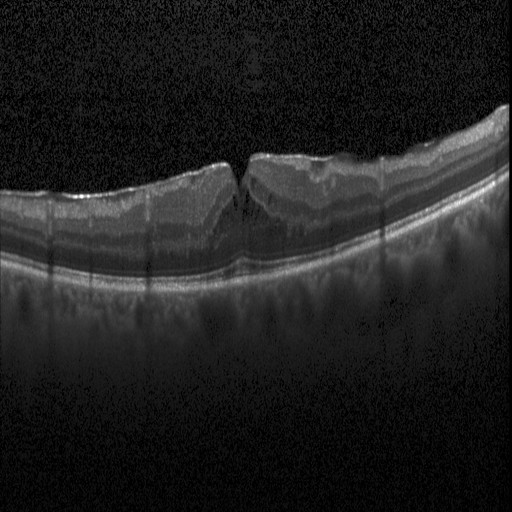

Retinal OCT cross-section — This B-scan demonstrates diabetic macular edema (DME).